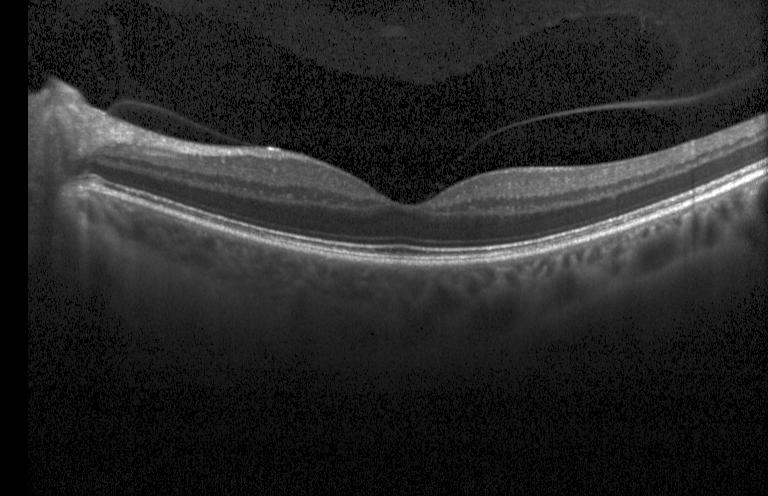 Spectral-domain OCT; OCT line scan. No choroidal neovascularization, diabetic macular edema, or drusen.